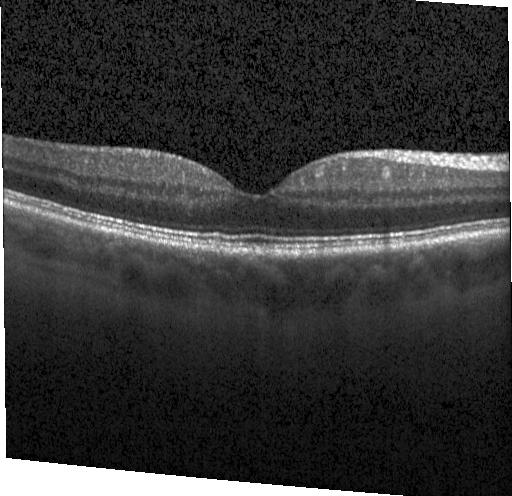

OCT B-scan
Diagnosis: no CNV, DME, or drusen.